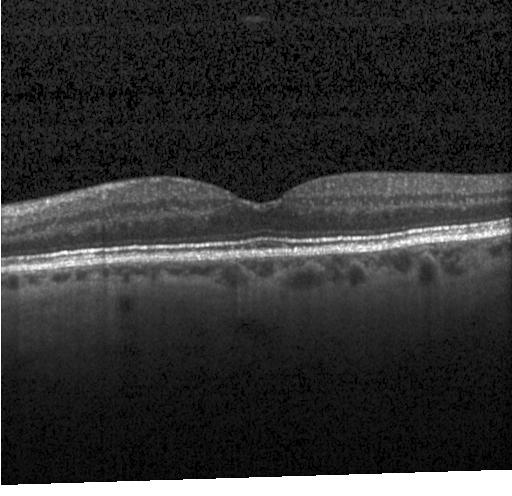

SD-OCT, instrument: Heidelberg Spectralis, optical coherence tomography scan — Neither CNV, DME, nor drusen.